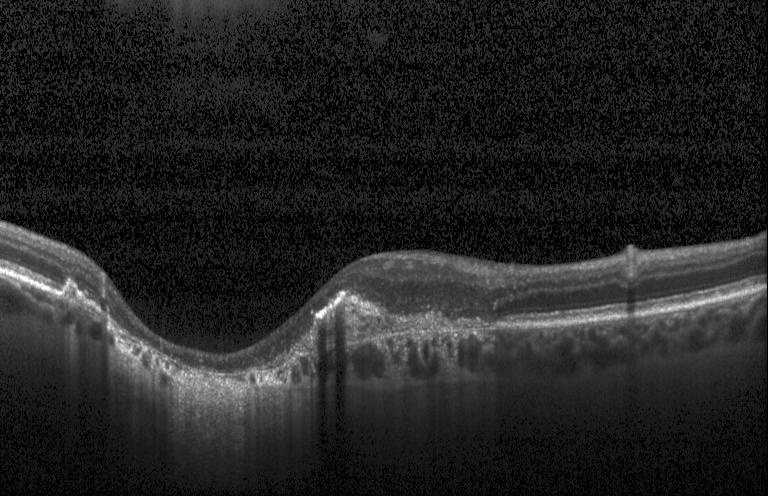

Finding: choroidal neovascularization (CNV).